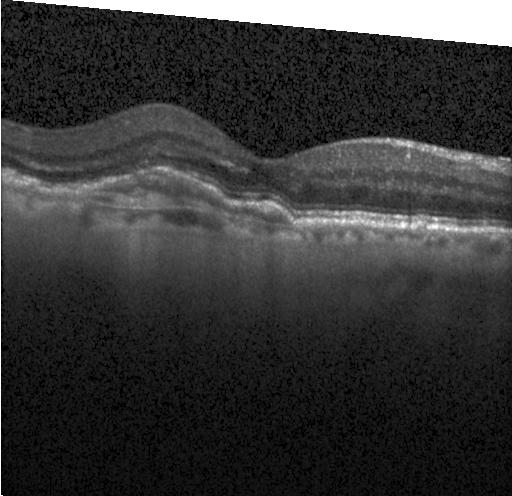 Spectral-domain OCT · centered on the fovea · instrument: Heidelberg Spectralis · optical coherence tomography scan. The scan shows CNV.